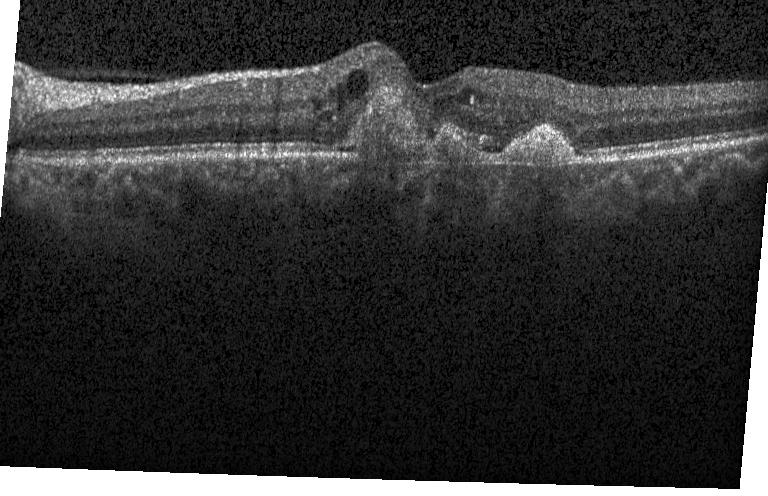 Macular scan · spectral-domain OCT · Heidelberg Spectralis OCT system · retinal OCT cross-section — Macular OCT: a choroidal neovascular membrane.